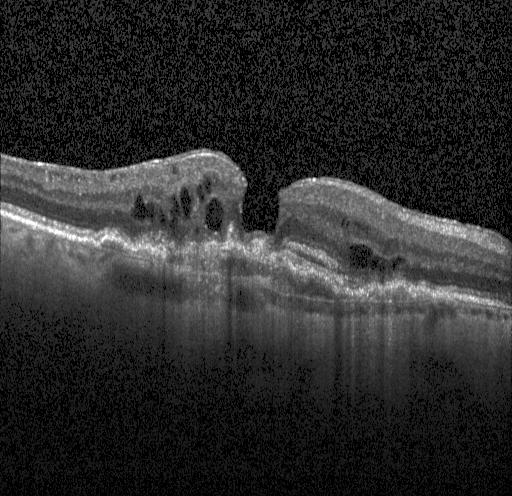 Choroidal neovascularization (CNV).